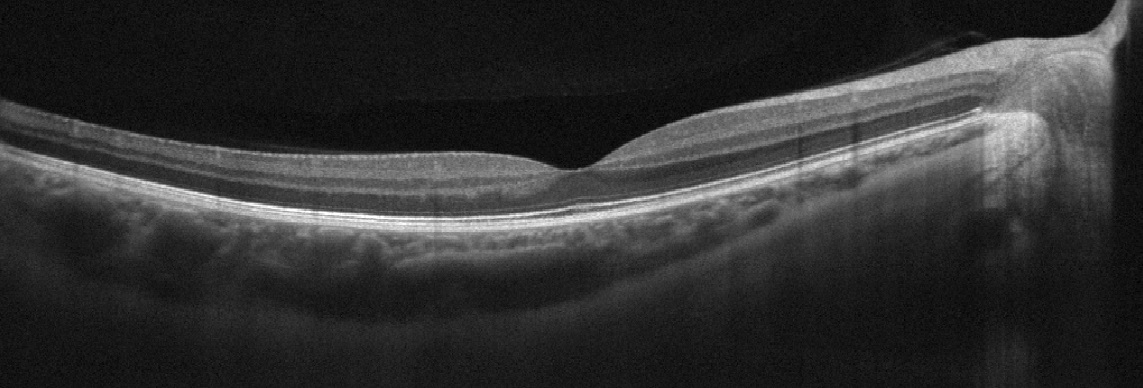

Acquired on an Optovue Avanti RTVue XR · optical coherence tomography scan — Assessment: no evidence of AMD, DME, ERM, RAO, RVO, or VID.